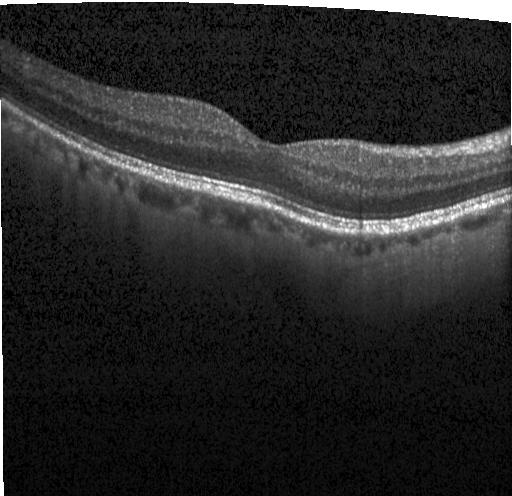
Through the macula, optical coherence tomography scan.
The scan shows no choroidal neovascularization, no diabetic macular edema, and no drusen.